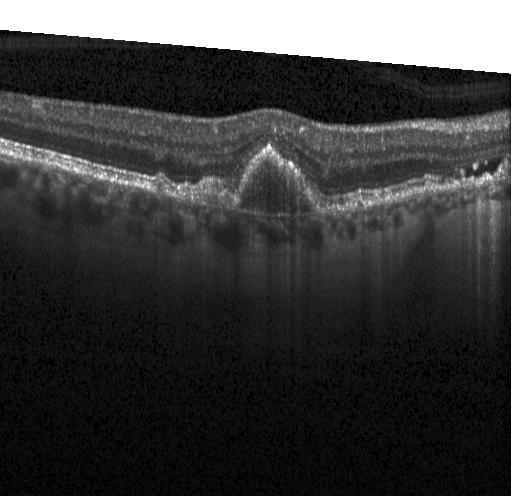
OCT finding: choroidal neovascularization (CNV).